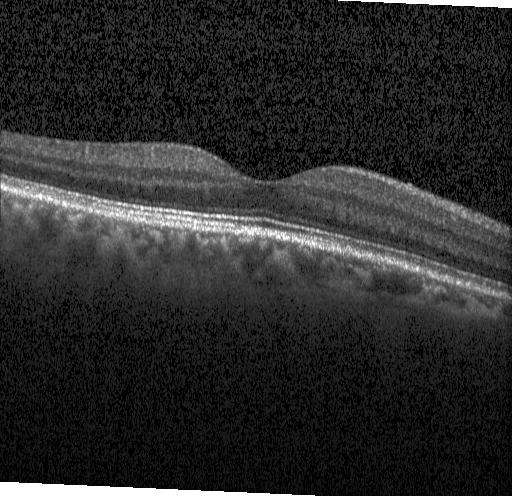
OCT B-scan showing no choroidal neovascularization, no diabetic macular edema, and no drusen.